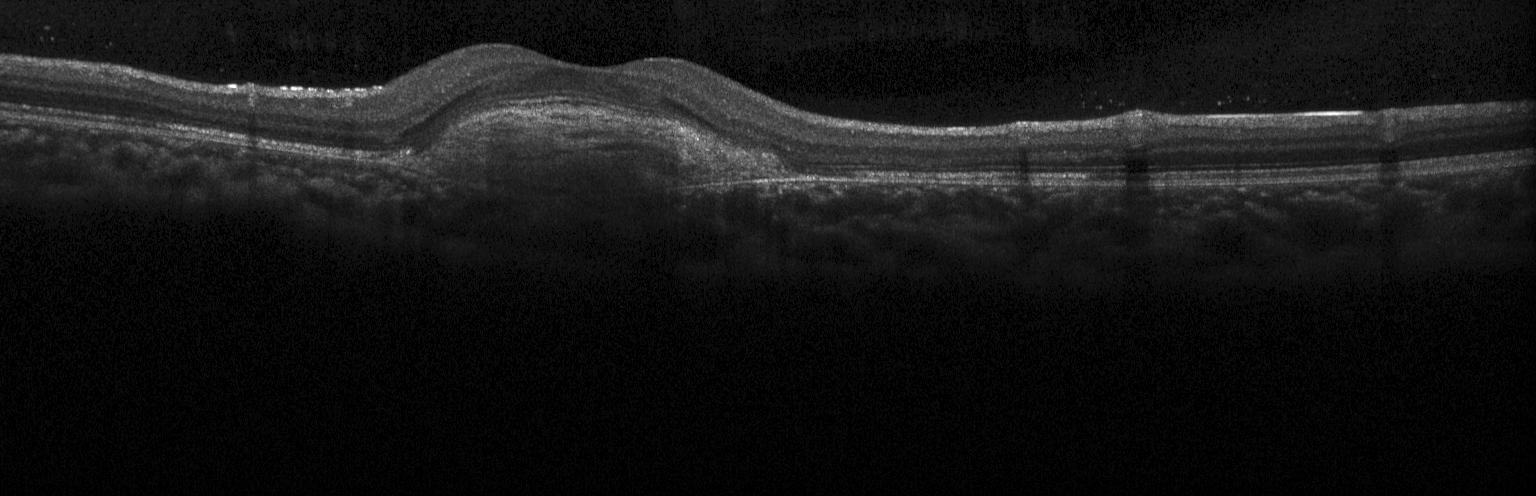

Finding: a choroidal neovascular membrane.